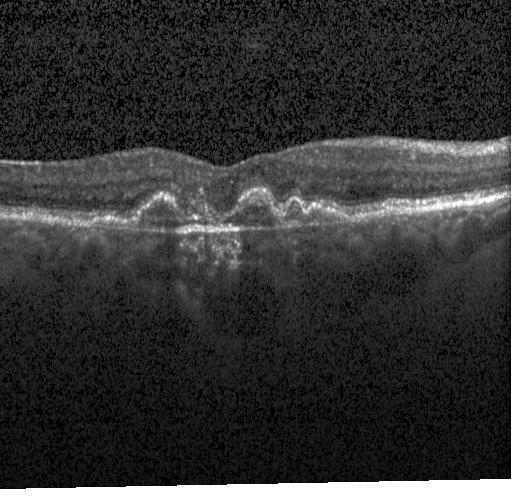 Optical coherence tomography scan.
The scan shows CNV.